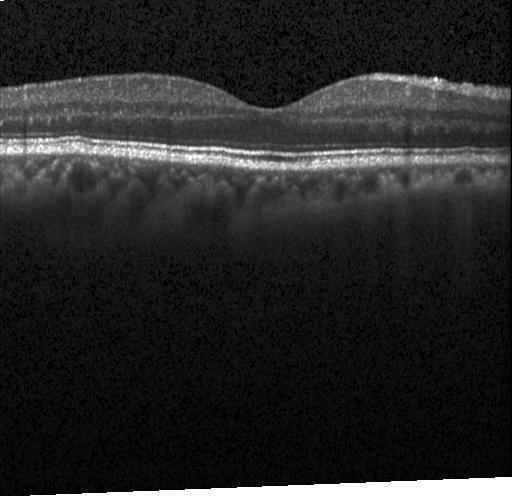 SD-OCT; instrument: Heidelberg Spectralis; macular scan; retinal OCT cross-section.
No evidence of CNV, DME, or drusen.